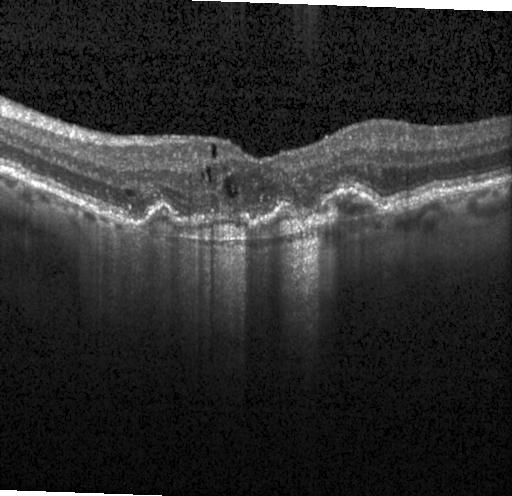 Macular OCT demonstrating CNV.